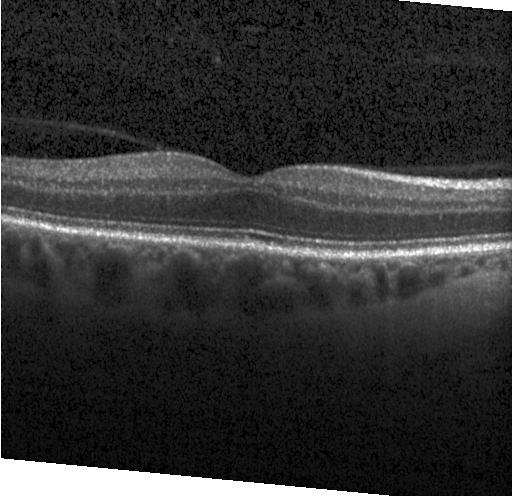

Retinal OCT B-scan — Assessment: neither choroidal neovascularization, diabetic macular edema, nor drusen.